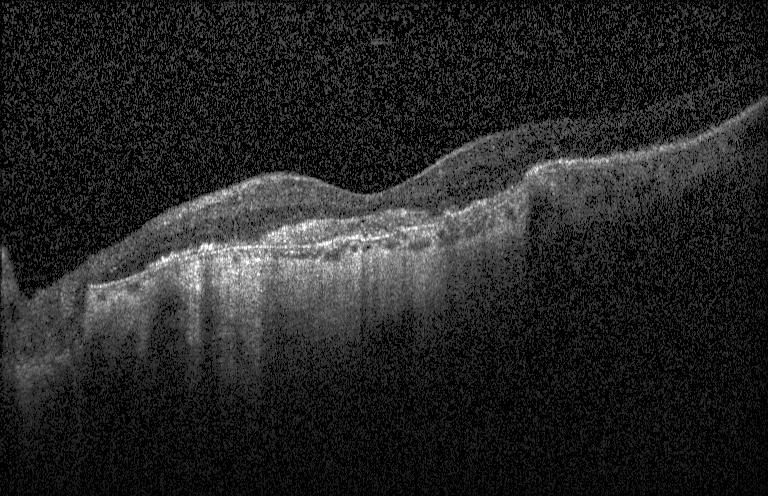

Retinal OCT cross-section showing choroidal neovascularization.